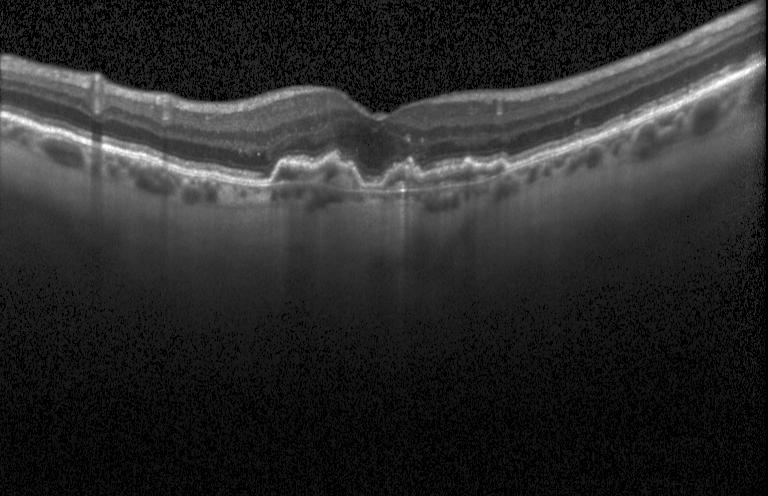 Macular OCT: CNV.